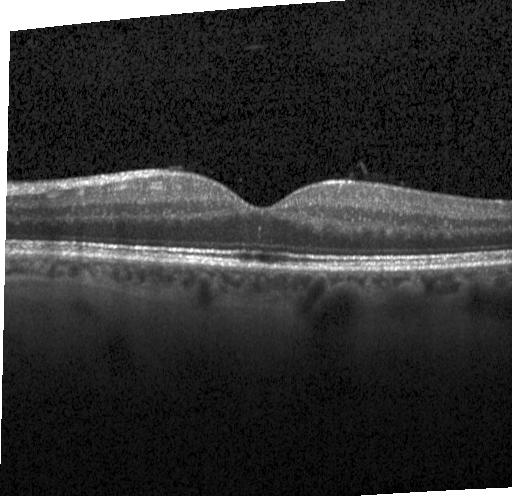 Instrument: Heidelberg Spectralis; horizontal scan through the fovea; optical coherence tomography B-scan; SD-OCT
Impression: no CNV, no DME, and no drusen.